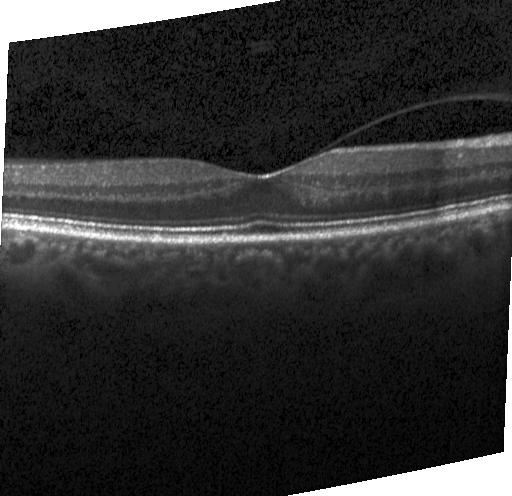

Retinal OCT cross-section showing no CNV, no DME, and no drusen.